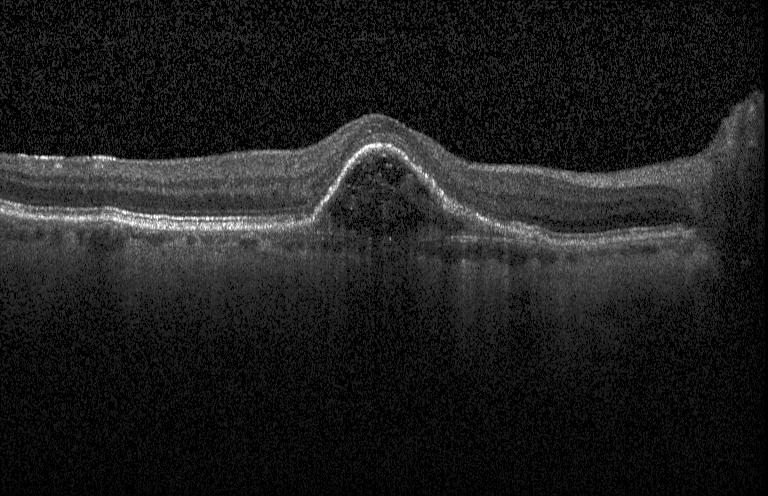

Retinal OCT B-scan — Finding: a choroidal neovascular membrane.